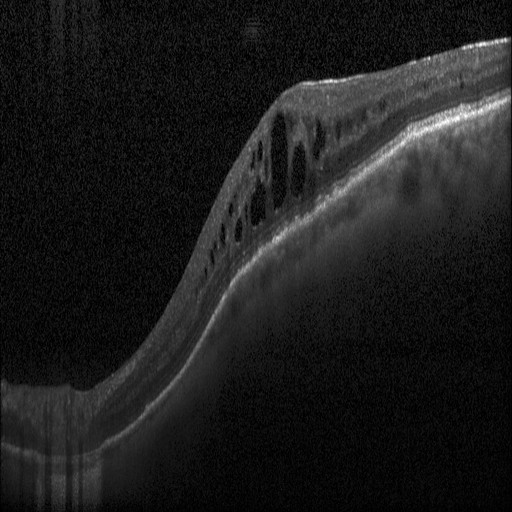
OCT B-scan. Macular scan. Instrument: Heidelberg Spectralis.
Diabetic macular edema.